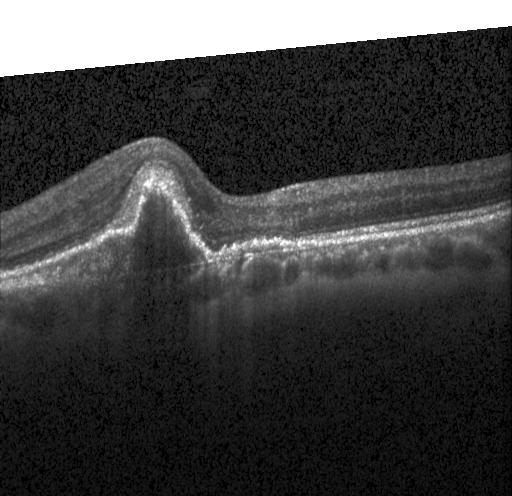 OCT line scan.
Diagnosis: a choroidal neovascular membrane.